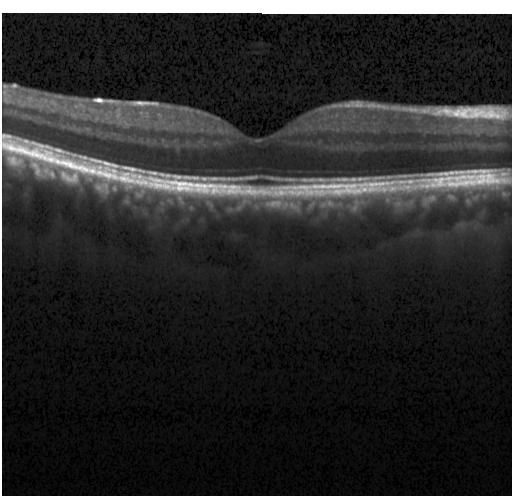
Acquired on a Heidelberg Spectralis. SD-OCT. Optical coherence tomography B-scan. Fovea-centered
Assessment: no choroidal neovascularization, diabetic macular edema, or drusen.